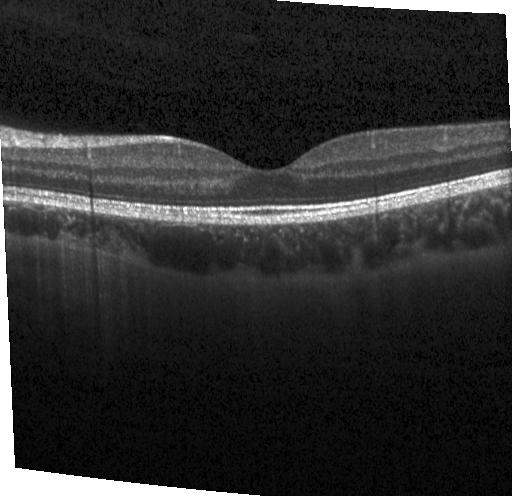

Spectral-domain OCT · OCT B-scan · centered on the fovea. Impression: neither choroidal neovascularization, diabetic macular edema, nor drusen.